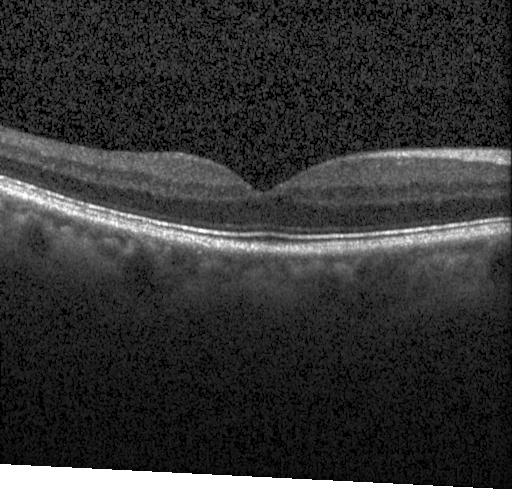 Retinal OCT cross-section. Spectral-domain OCT — OCT finding: no CNV, no DME, and no drusen.